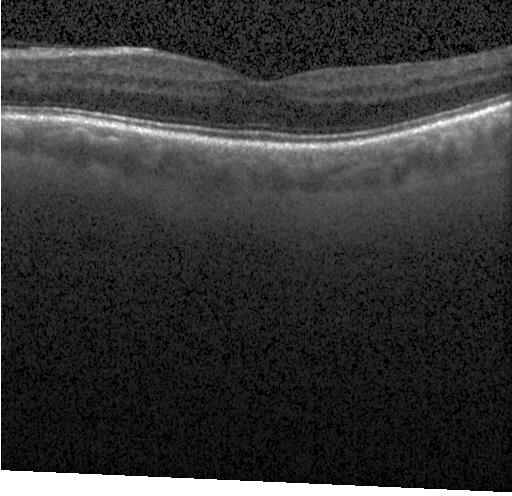 Heidelberg Spectralis OCT system, horizontal scan through the fovea, retinal OCT B-scan.
Finding: no choroidal neovascularization, diabetic macular edema, or drusen.